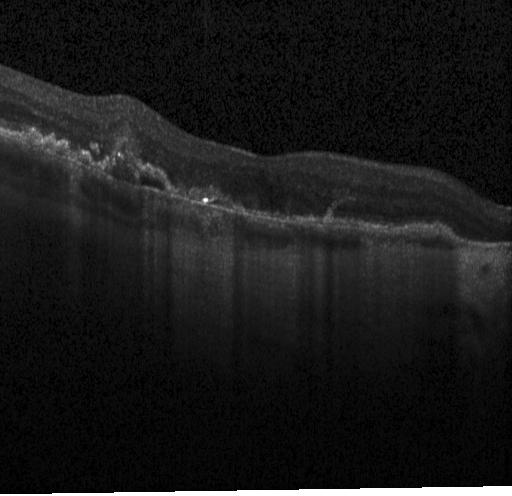

Impression: a choroidal neovascular membrane.